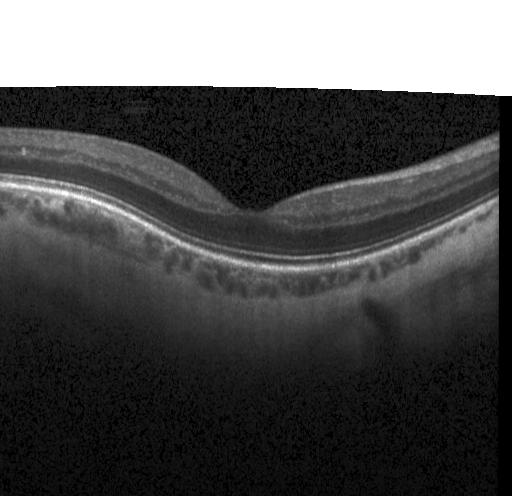 Impression: no evidence of choroidal neovascularization, diabetic macular edema, or drusen.